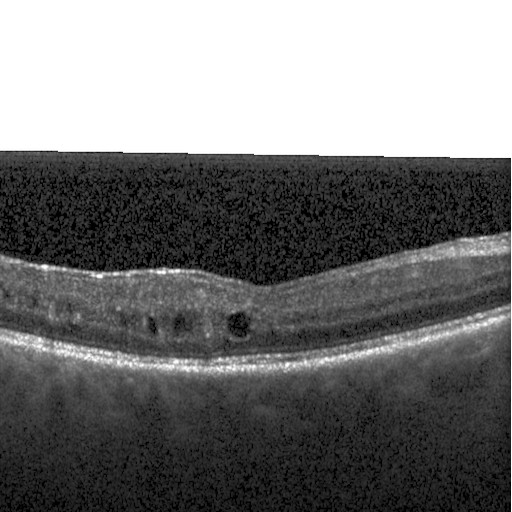
Optical coherence tomography scan — Finding: diabetic macular edema.